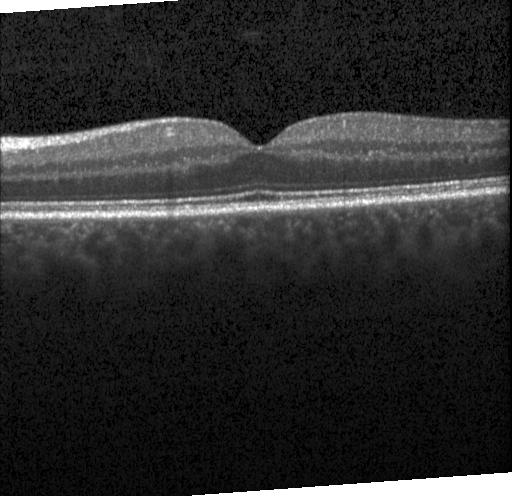
Retinal OCT B-scan, Heidelberg Spectralis. Impression: no CNV, no DME, and no drusen.